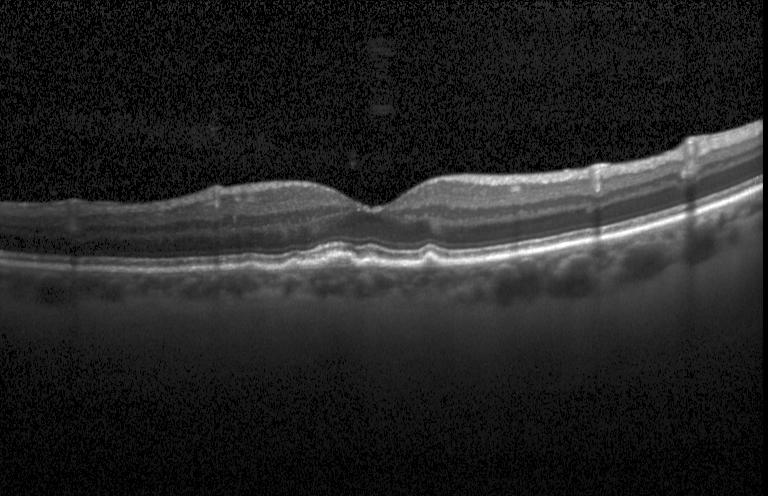

OCT B-scan; macular scan. Macular OCT: multiple drusen.